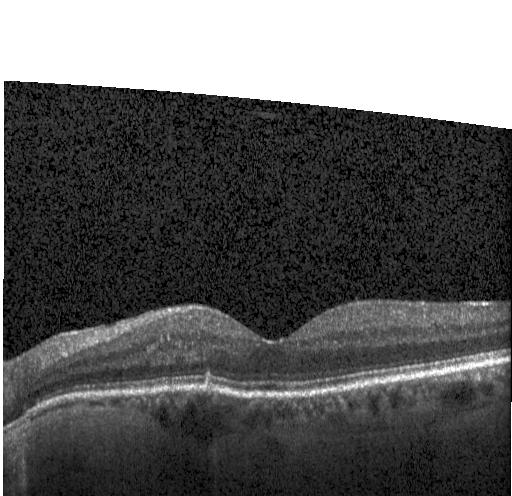

Sub-RPE drusenoid deposits.